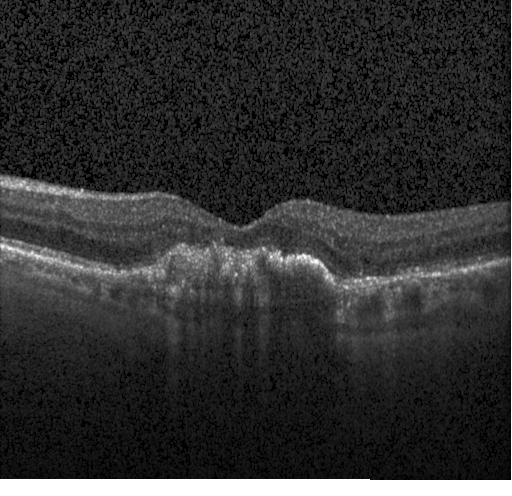

OCT B-scan — Dx: a choroidal neovascular membrane.